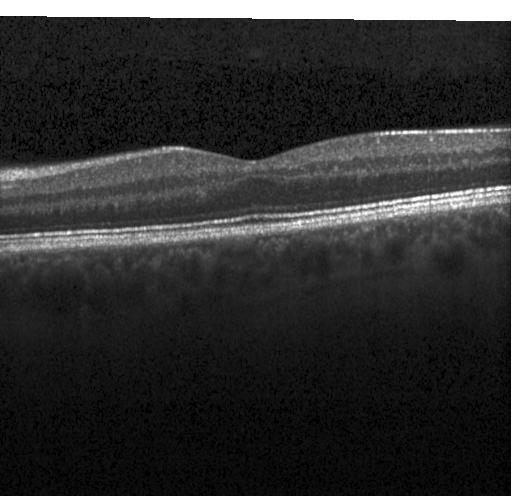 Impression: no CNV, no DME, and no drusen.